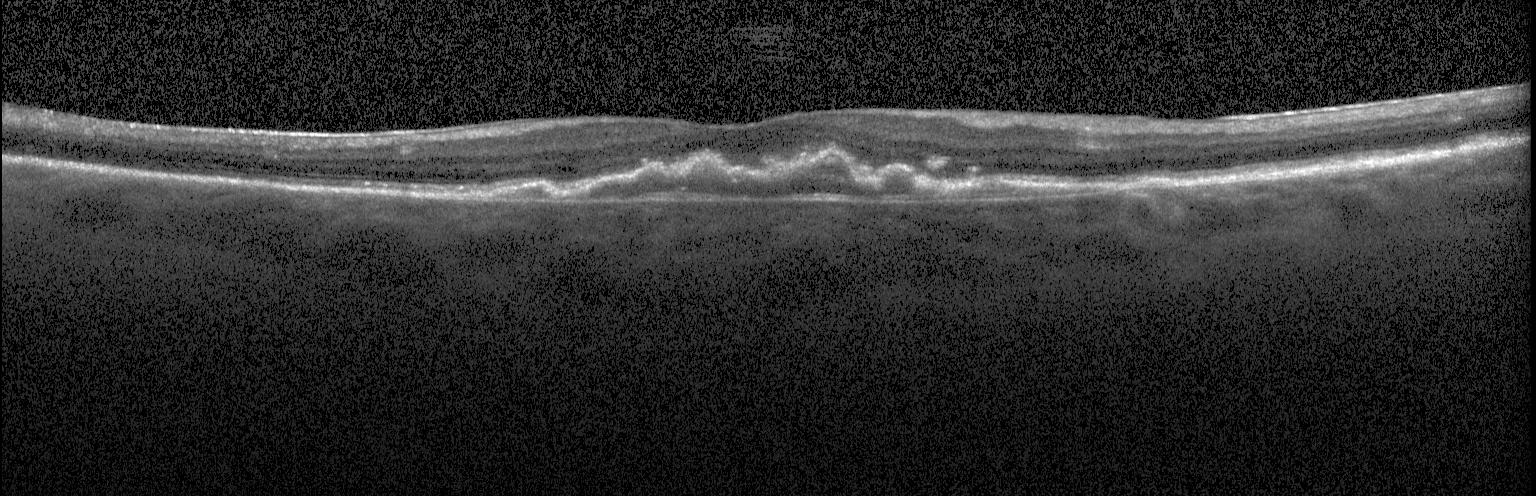 Finding: CNV.